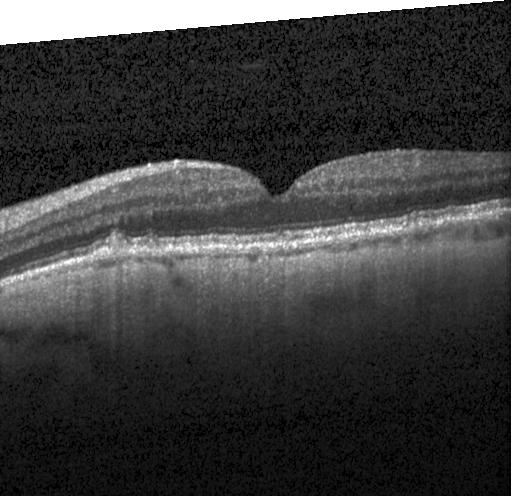
Impression: drusen.